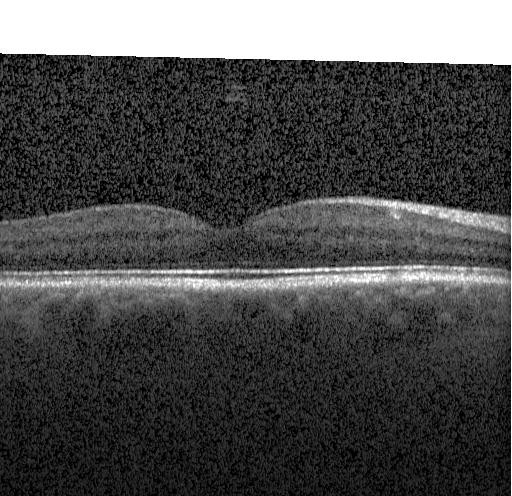

Retinal OCT B-scan.
Diagnosis: no CNV, no DME, and no drusen.